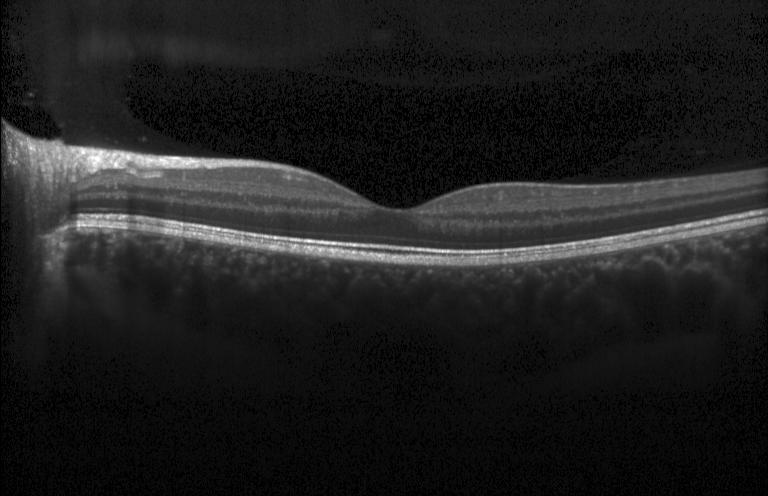
Acquired on a Heidelberg Spectralis, optical coherence tomography B-scan. Assessment: no CNV, DME, or drusen.